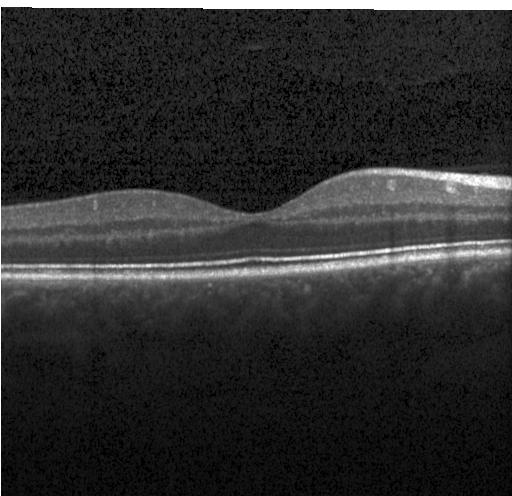 This B-scan demonstrates no choroidal neovascularization, no diabetic macular edema, and no drusen.